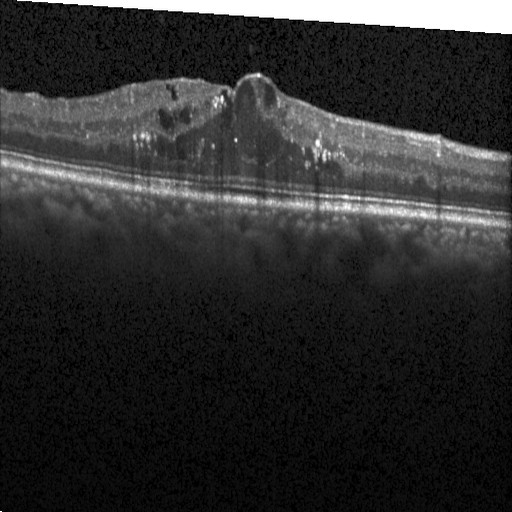 Assessment: diabetic macular edema.